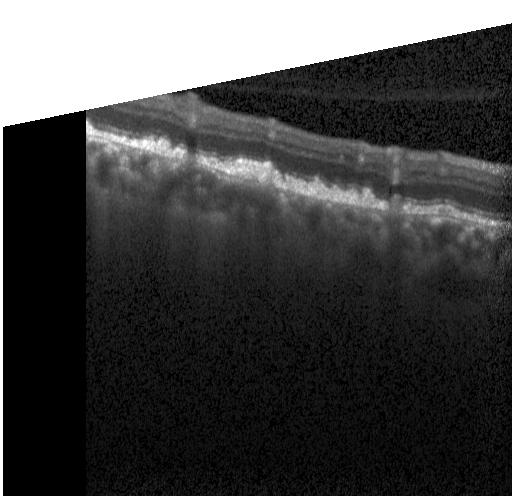
Retinal OCT B-scan · centered on the fovea · spectral-domain optical coherence tomography · instrument: Heidelberg Spectralis.
Impression: sub-RPE drusenoid deposits.